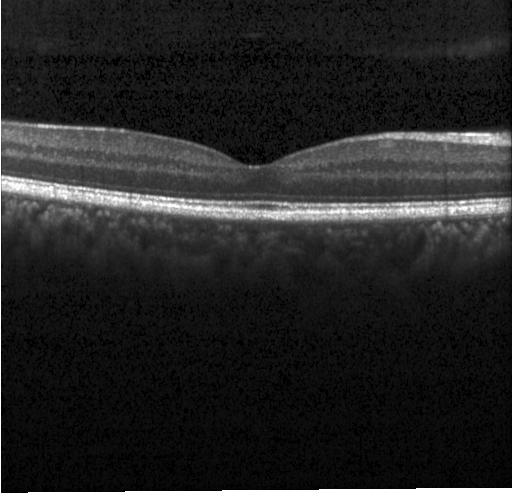 Spectral-domain optical coherence tomography · macular scan · optical coherence tomography scan — Assessment: no choroidal neovascularization, diabetic macular edema, or drusen.